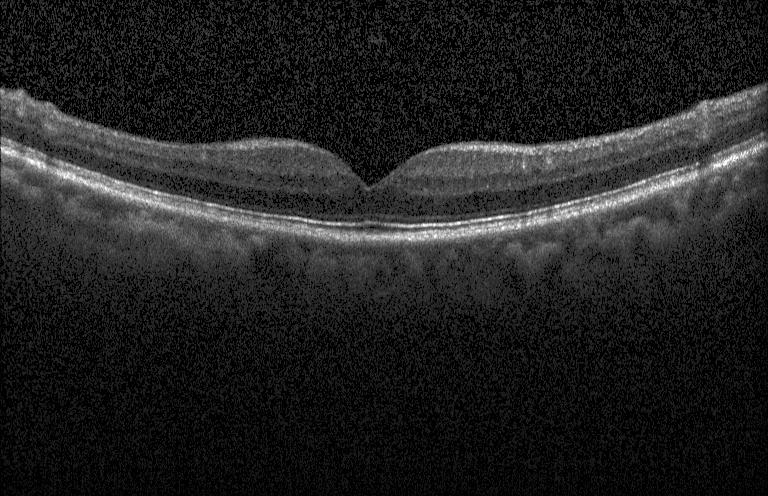
Spectral-domain OCT · retinal OCT cross-section. Impression: neither choroidal neovascularization, diabetic macular edema, nor drusen.